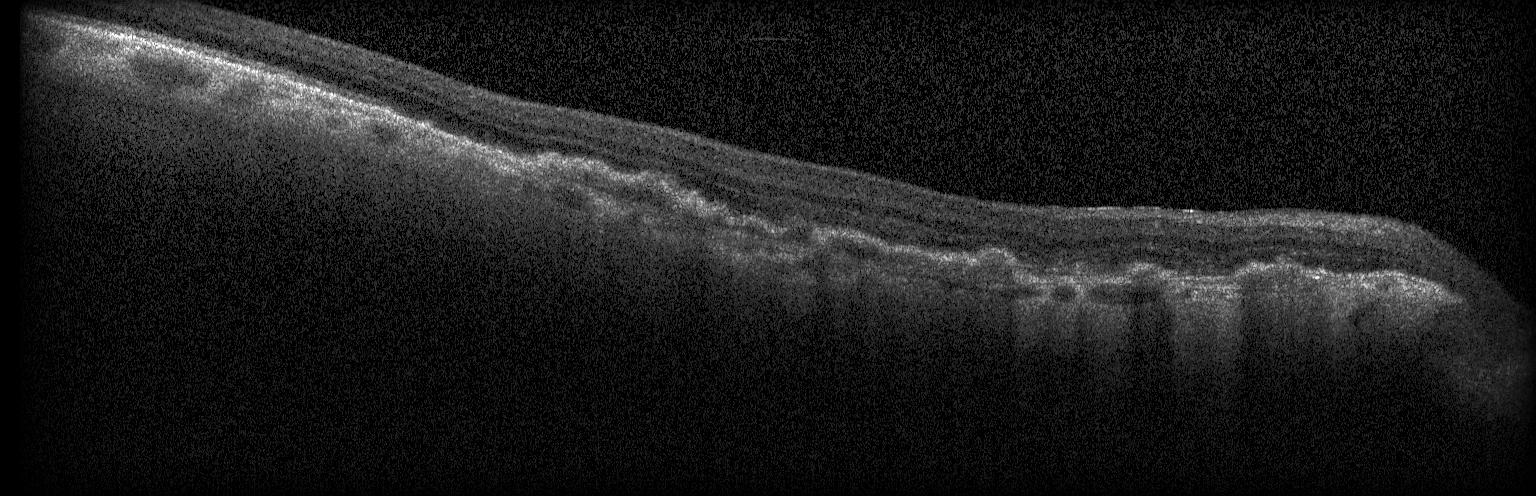

Impression: choroidal neovascularization.